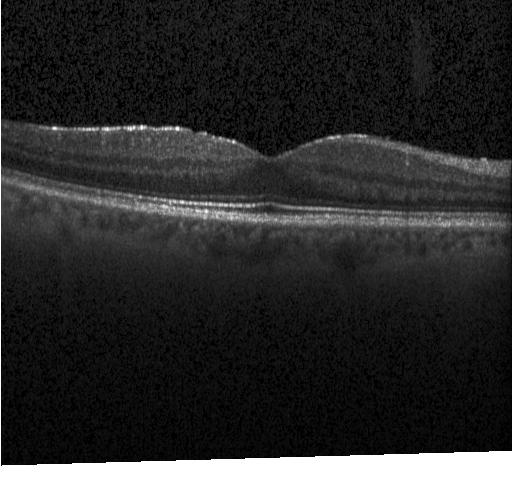

Impression: no CNV, DME, or drusen.